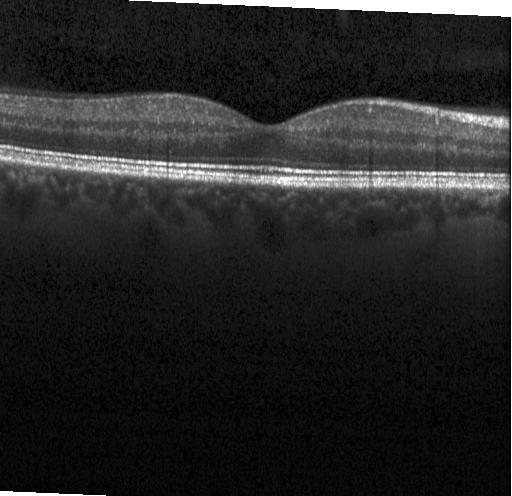
Centered on the fovea · optical coherence tomography B-scan
Assessment: no choroidal neovascularization, diabetic macular edema, or drusen.